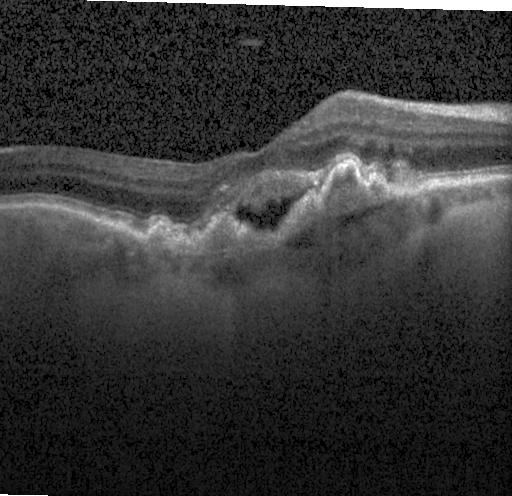

Spectral-domain optical coherence tomography · macular scan · Heidelberg Spectralis OCT system · optical coherence tomography scan — Impression: choroidal neovascularization (CNV).